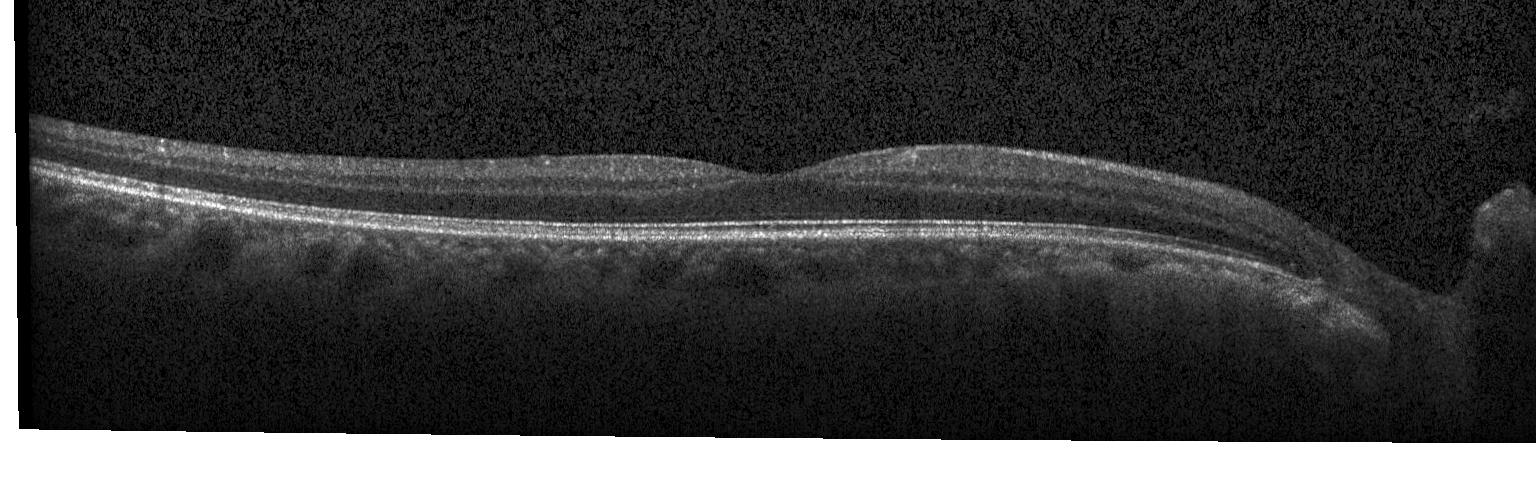 Finding: no evidence of choroidal neovascularization, diabetic macular edema, or drusen.